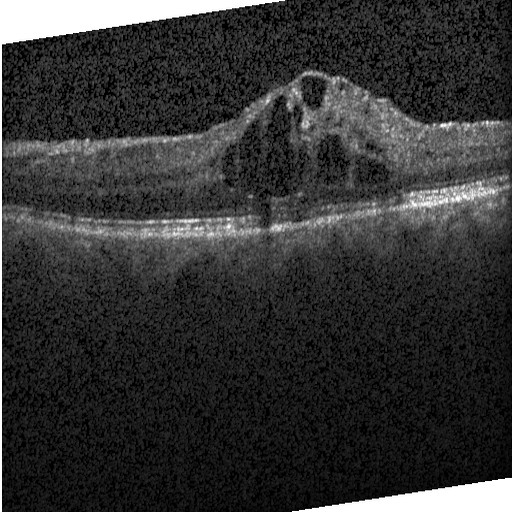
SD-OCT · retinal OCT B-scan — Dx: diabetic macular edema (DME).